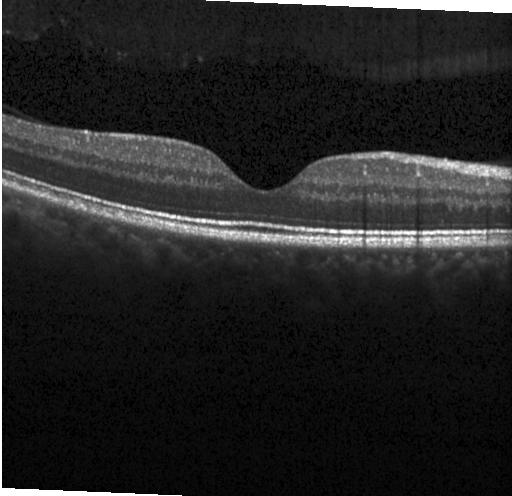
Retinal OCT B-scan · macular scan · Heidelberg Spectralis · spectral-domain optical coherence tomography — OCT finding: neither choroidal neovascularization, diabetic macular edema, nor drusen.